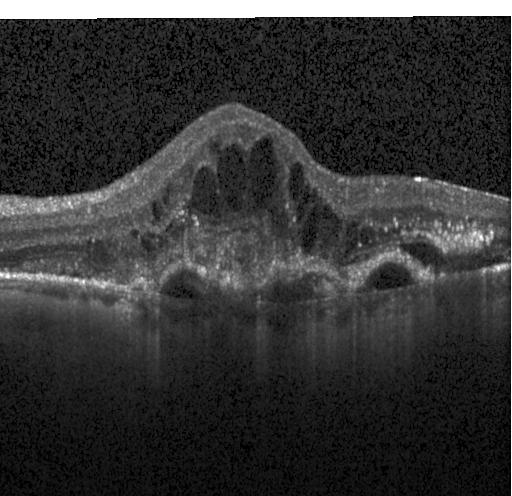

Retinal OCT B-scan. A choroidal neovascular membrane.